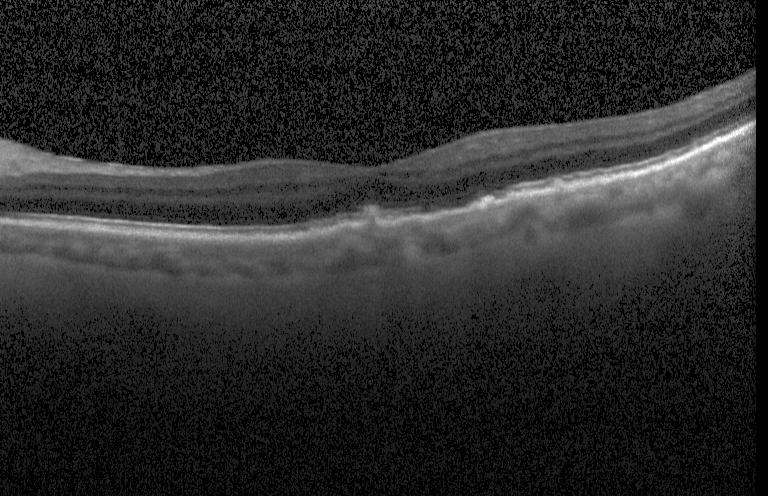 OCT line scan.
Assessment: sub-RPE drusenoid deposits.